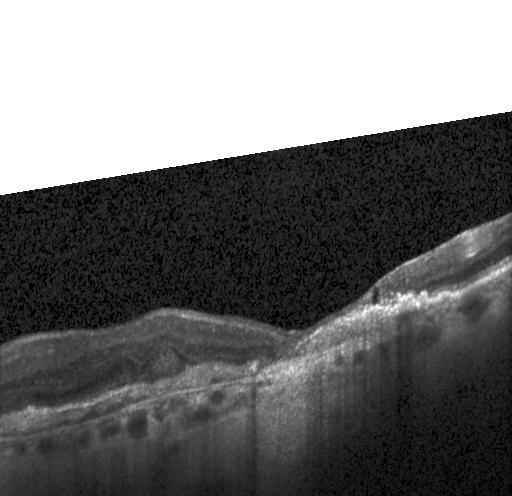

Spectral-domain OCT, retinal OCT B-scan, instrument: Heidelberg Spectralis, horizontal scan through the fovea. This B-scan demonstrates choroidal neovascularization (CNV).